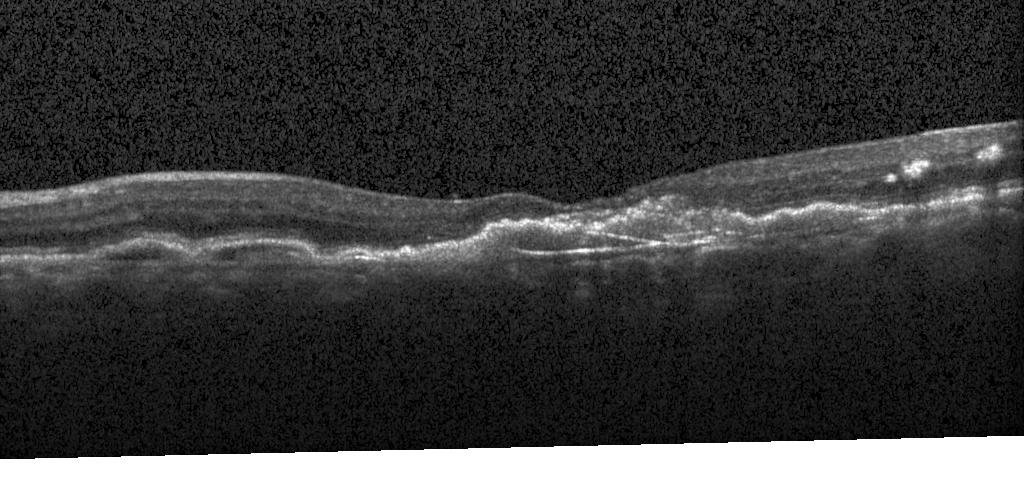

Retinal OCT B-scan.
Finding: choroidal neovascularization.